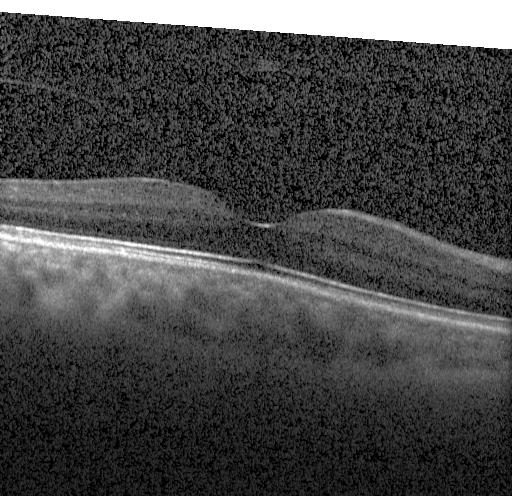

SD-OCT; Heidelberg Spectralis; centered on the fovea; retinal OCT B-scan.
Diagnosis: no choroidal neovascularization, no diabetic macular edema, and no drusen.